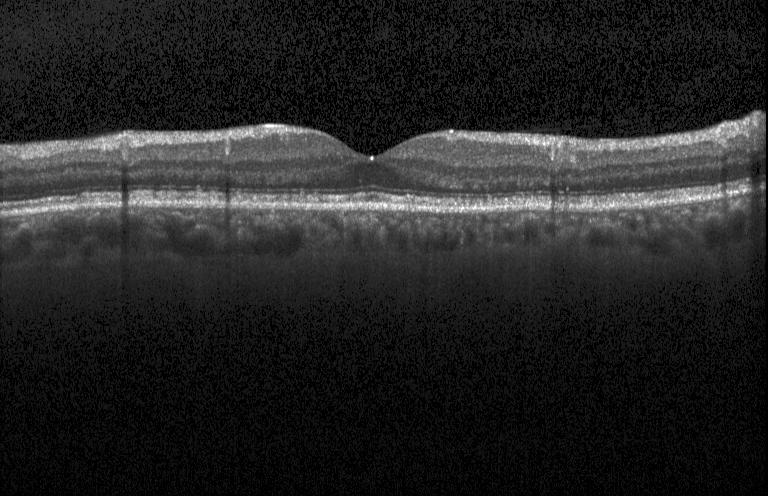

Centered on the fovea · OCT B-scan
The scan shows no choroidal neovascularization, no diabetic macular edema, and no drusen.